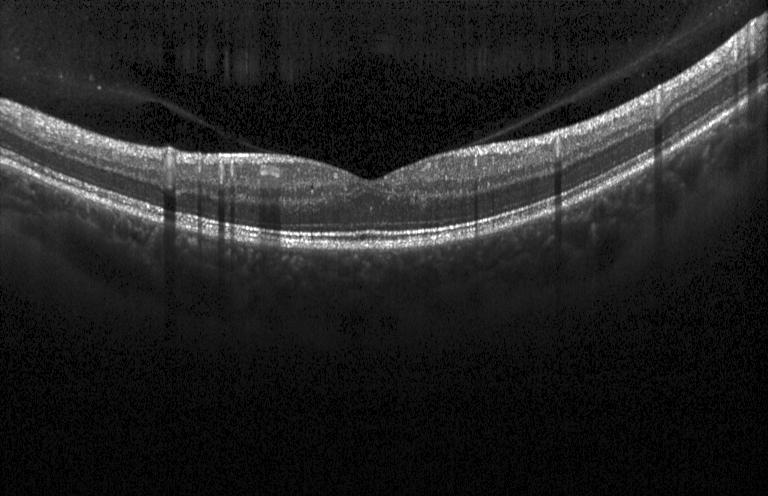
Diagnosis: no choroidal neovascularization, diabetic macular edema, or drusen.